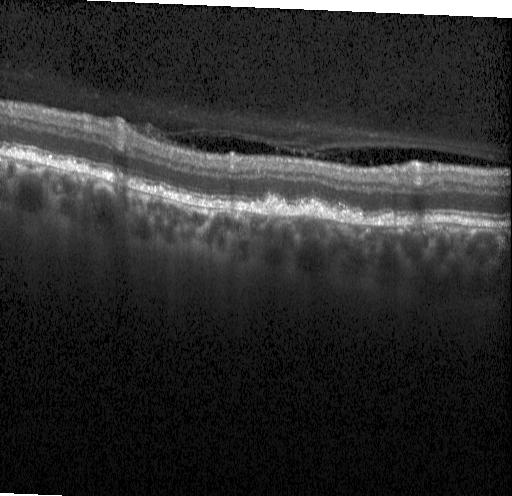 Retinal OCT B-scan; centered on the fovea; SD-OCT.
Assessment: multiple drusen.